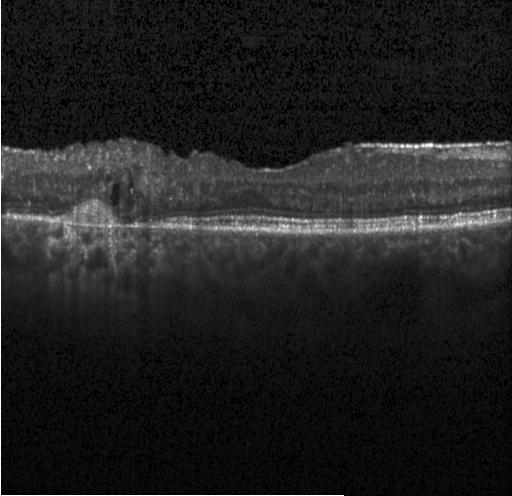
Centered on the fovea. Heidelberg Spectralis OCT system. Retinal OCT B-scan. Spectral-domain OCT.
Finding: choroidal neovascularization (CNV).